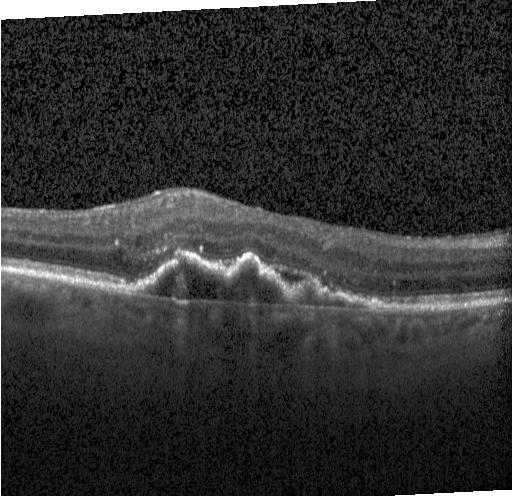

Spectral-domain OCT. Optical coherence tomography scan. Heidelberg Spectralis. Impression: choroidal neovascularization.